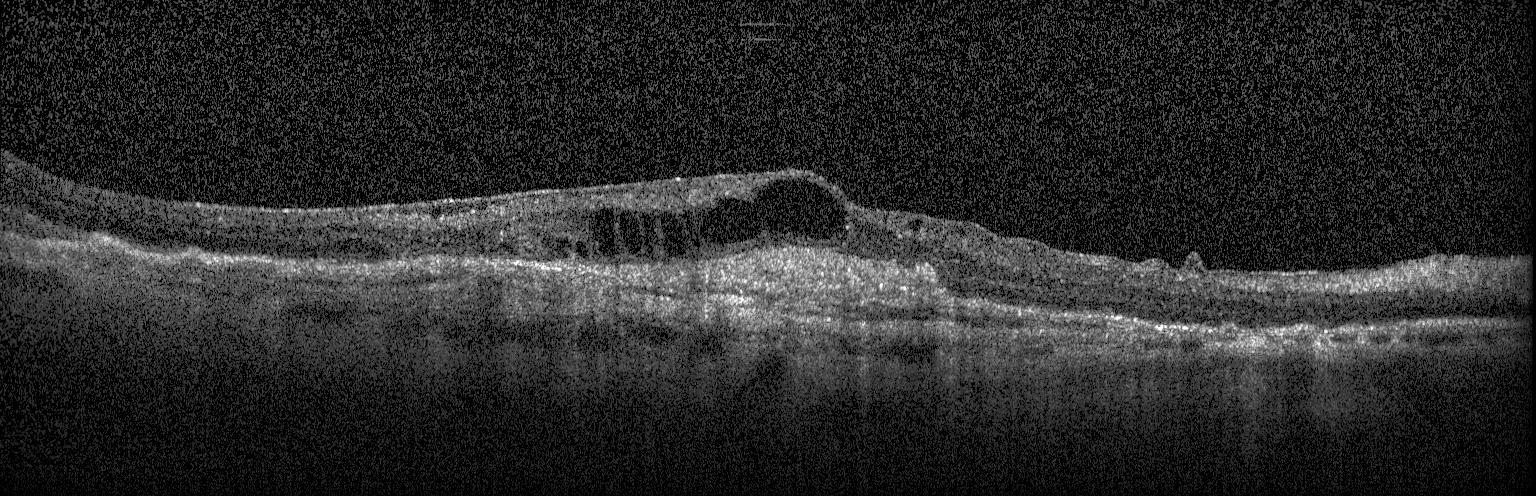
This B-scan demonstrates choroidal neovascularization.